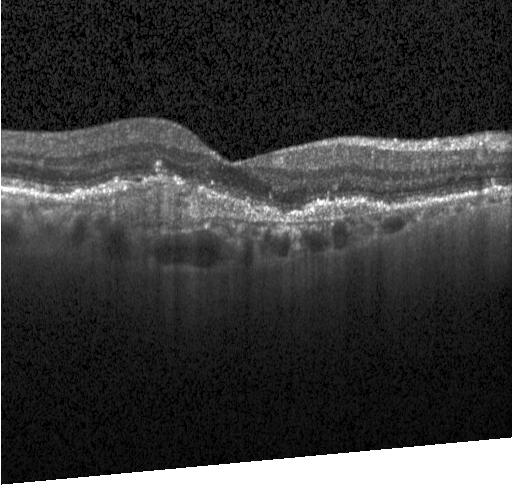
OCT line scan · horizontal scan through the fovea · Heidelberg Spectralis · SD-OCT. Diagnosis: choroidal neovascularization (CNV).